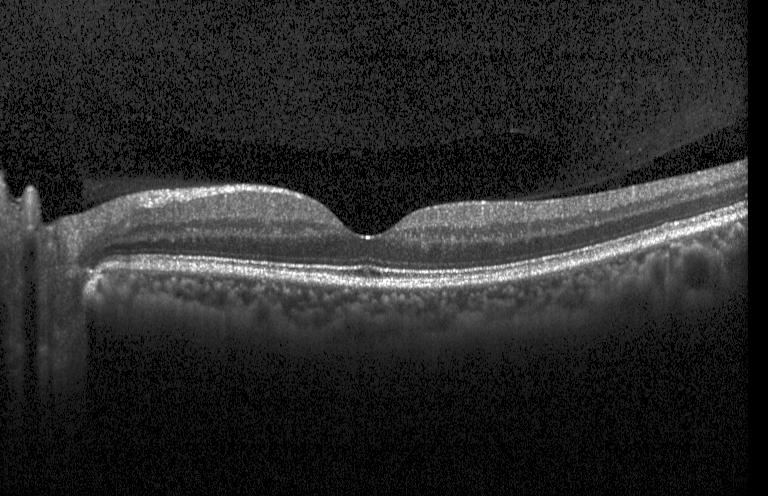

SD-OCT; OCT B-scan — Impression: no choroidal neovascularization, diabetic macular edema, or drusen.